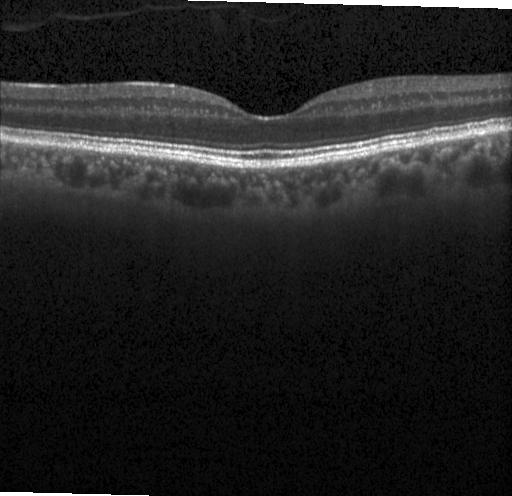

Heidelberg Spectralis OCT system. OCT line scan. Spectral-domain optical coherence tomography — Impression: no CNV, no DME, and no drusen.